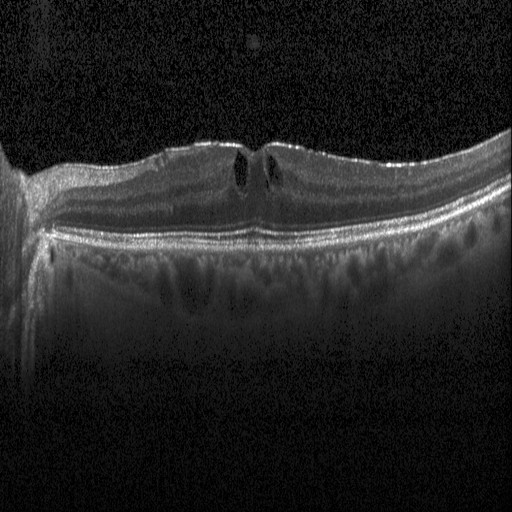 DME.